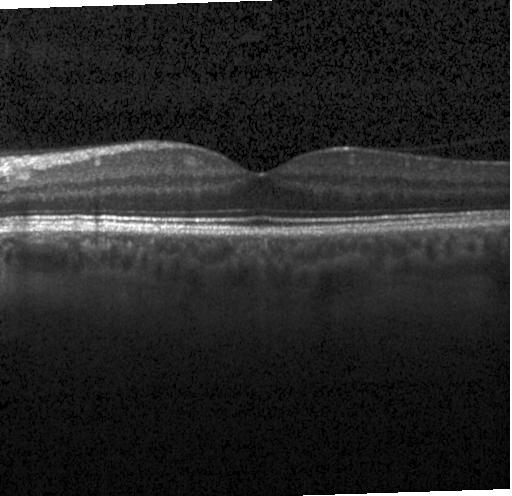 Spectral-domain OCT, optical coherence tomography B-scan, macular scan. Diagnosis: no CNV, no DME, and no drusen.